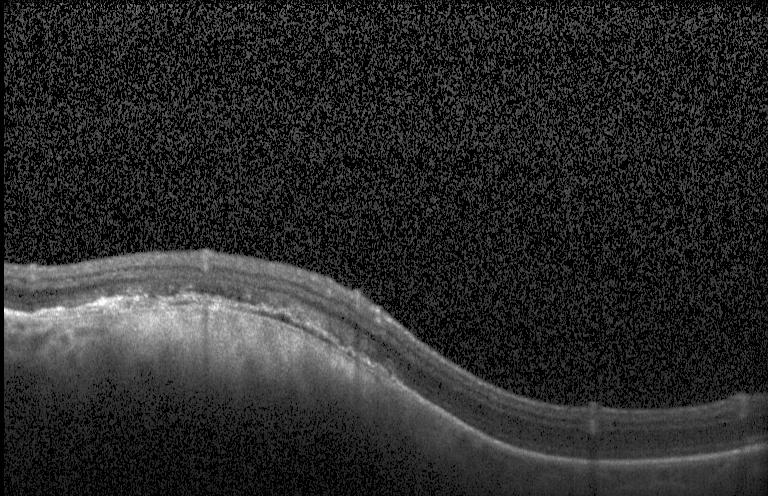 Through the macula. OCT B-scan. SD-OCT. The scan shows CNV.